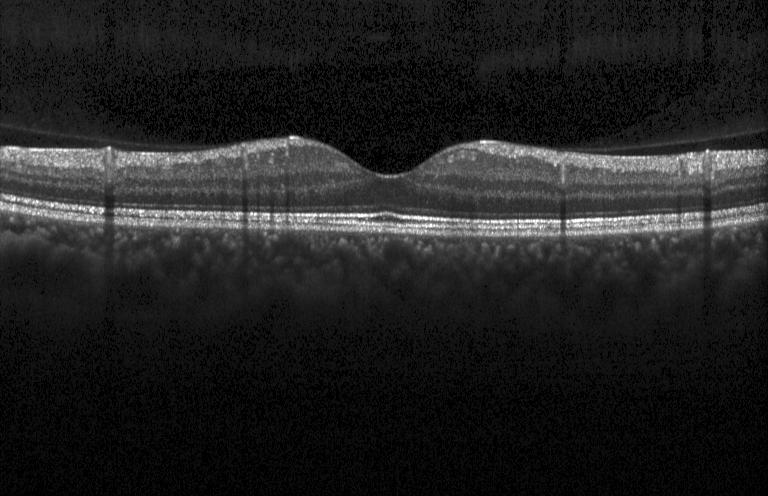 Retinal OCT cross-section — Impression: no choroidal neovascularization, diabetic macular edema, or drusen.